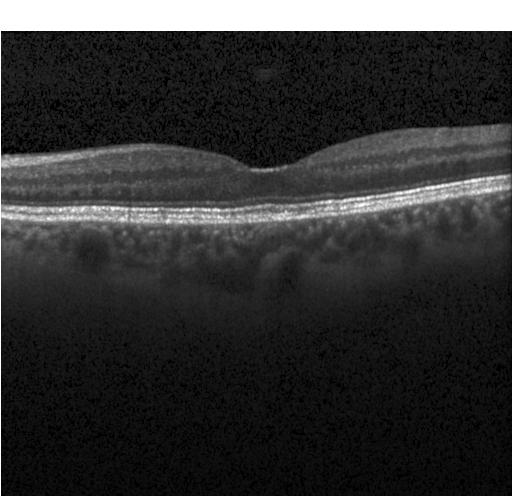

Spectral-domain OCT · optical coherence tomography scan — Assessment: no evidence of CNV, DME, or drusen.